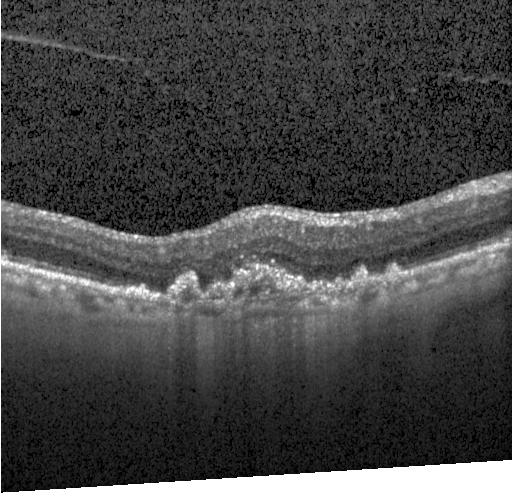
Acquired on a Heidelberg Spectralis. Through the macula. Spectral-domain OCT. Optical coherence tomography scan. OCT finding: a choroidal neovascular membrane.